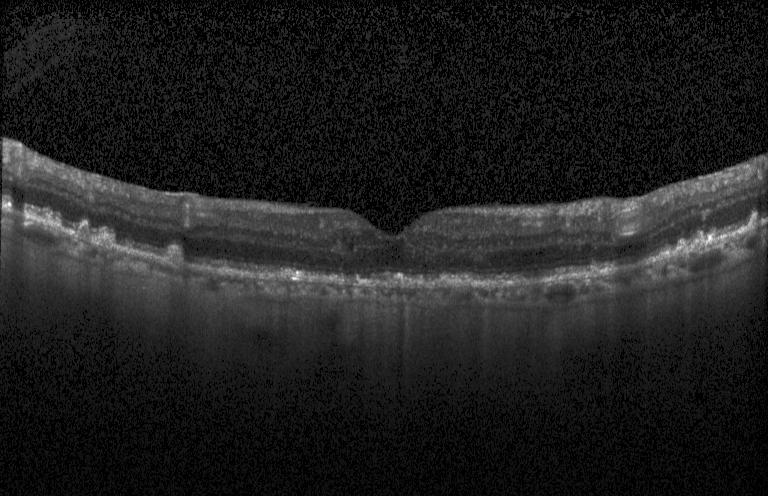
OCT B-scan showing a choroidal neovascular membrane.